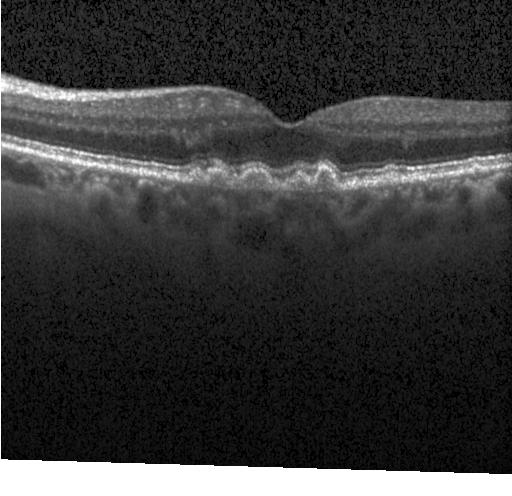

Spectral-domain OCT, horizontal scan through the fovea, instrument: Heidelberg Spectralis, retinal OCT cross-section. Dx: drusen.